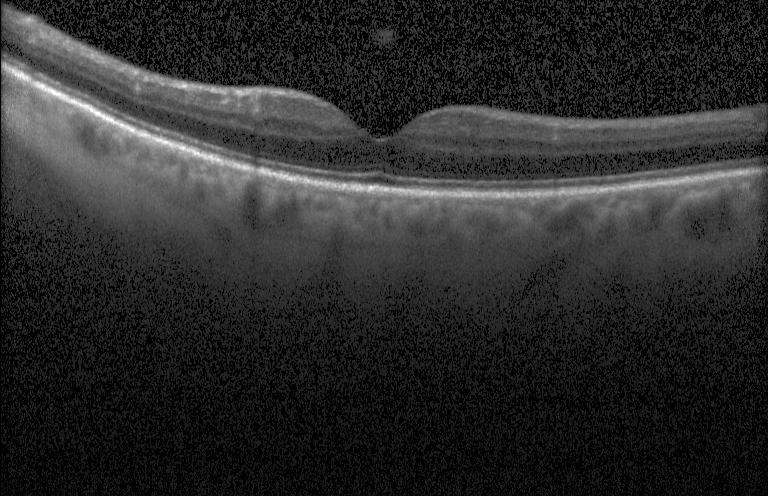

Optical coherence tomography scan; acquired on a Heidelberg Spectralis; spectral-domain OCT. Finding: no evidence of choroidal neovascularization, diabetic macular edema, or drusen.